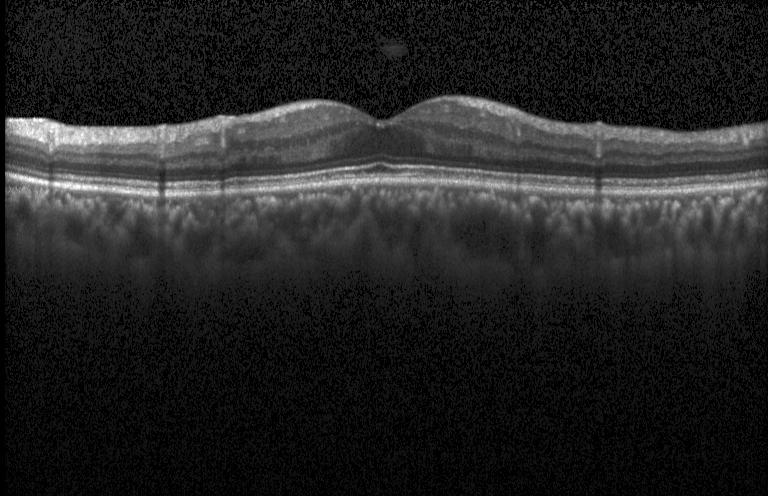

Retinal OCT cross-section showing no CNV, no DME, and no drusen.